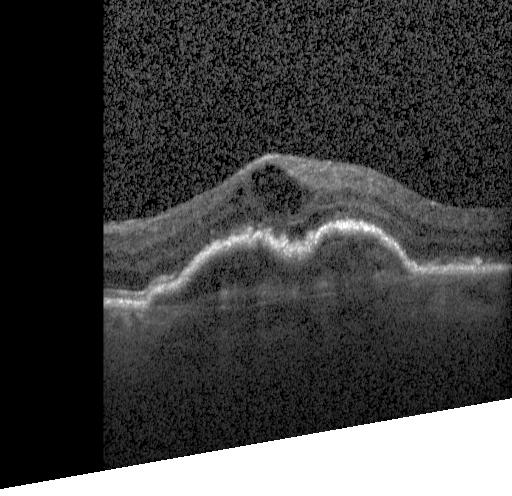
Optical coherence tomography scan. Instrument: Heidelberg Spectralis. Spectral-domain optical coherence tomography. Through the macula — CNV.